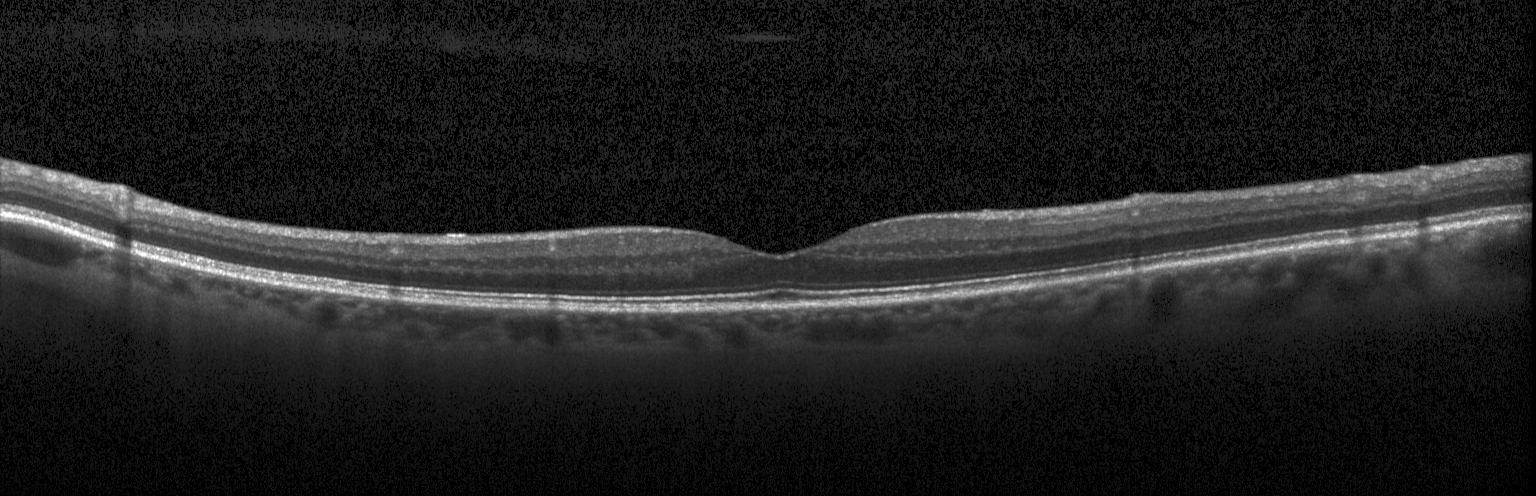

Centered on the fovea. SD-OCT. OCT line scan. Instrument: Heidelberg Spectralis — This B-scan demonstrates no CNV, no DME, and no drusen.